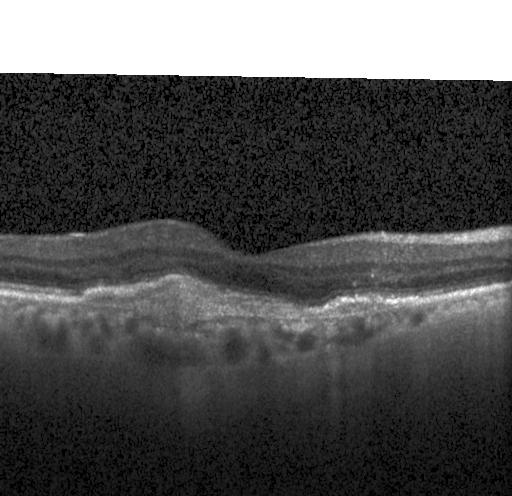 Spectral-domain OCT; instrument: Heidelberg Spectralis; OCT B-scan; centered on the fovea — Choroidal neovascularization.